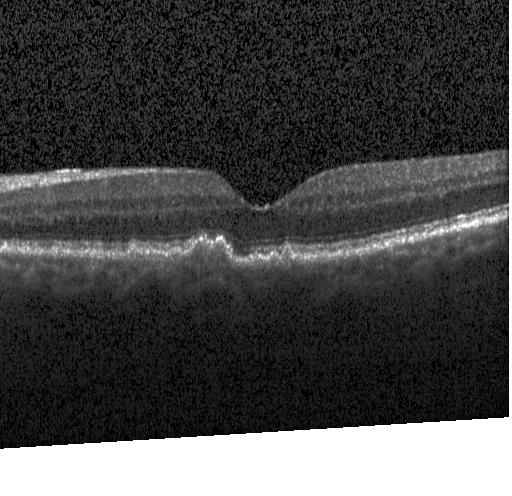

Finding: drusen.